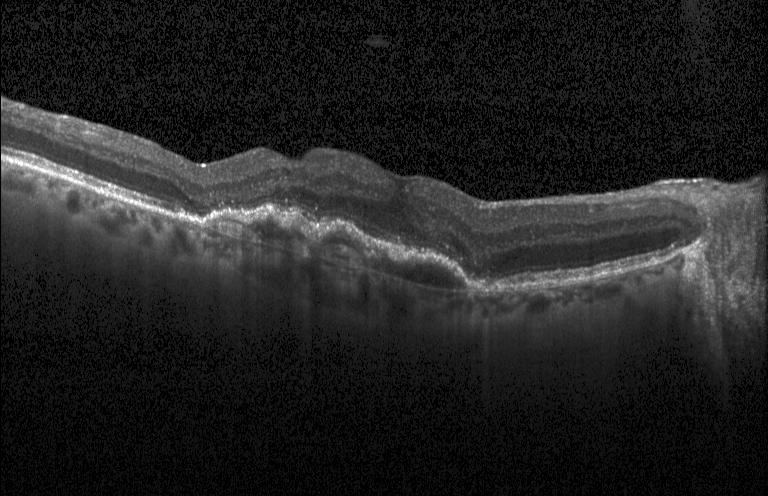 OCT B-scan. CNV.